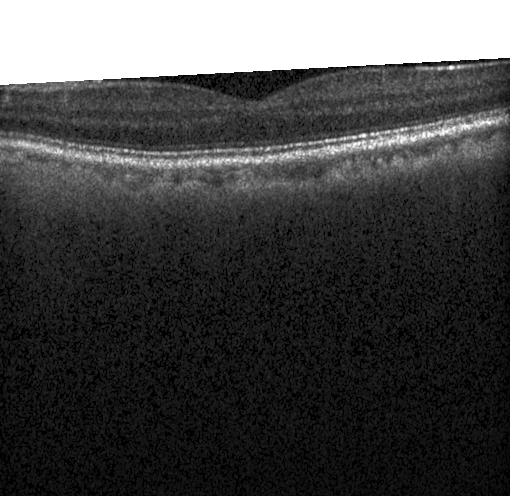
OCT B-scan. Dx: neither choroidal neovascularization, diabetic macular edema, nor drusen.